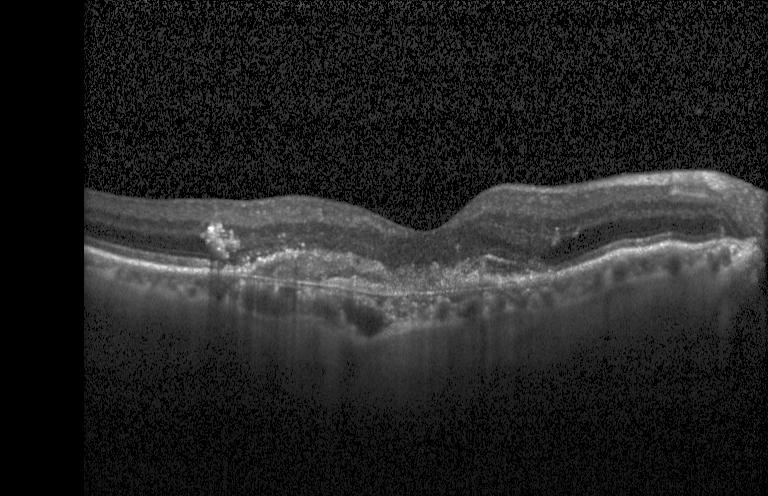 OCT line scan
This B-scan demonstrates a choroidal neovascular membrane.